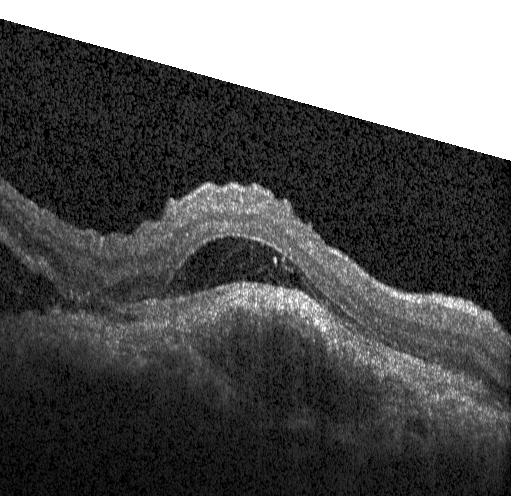
Macular OCT demonstrating CNV.